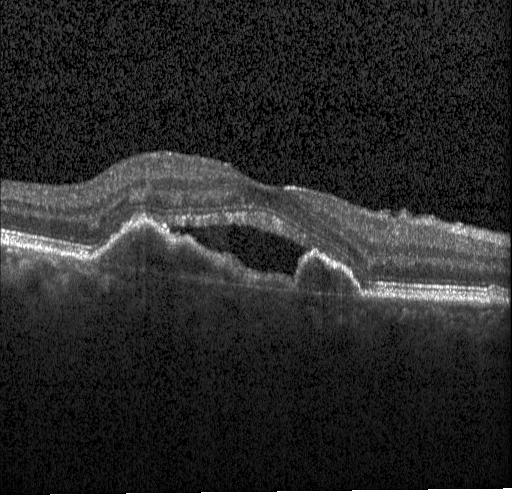
Finding: choroidal neovascularization (CNV).